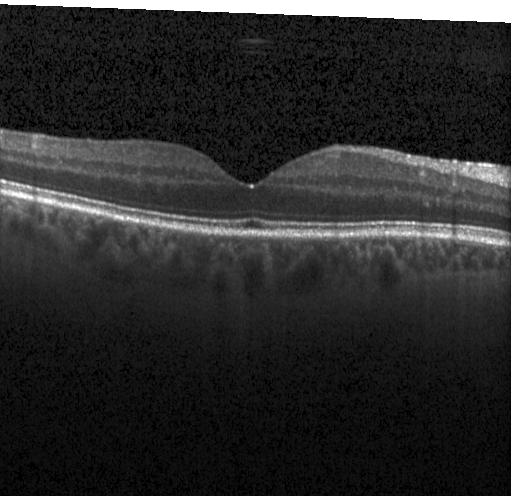
OCT B-scan.
No evidence of CNV, DME, or drusen.